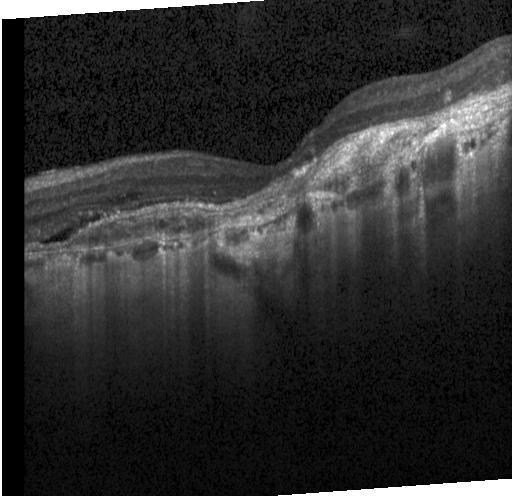
Through the macula; Heidelberg Spectralis; spectral-domain optical coherence tomography; OCT B-scan.
Macular OCT: choroidal neovascularization.